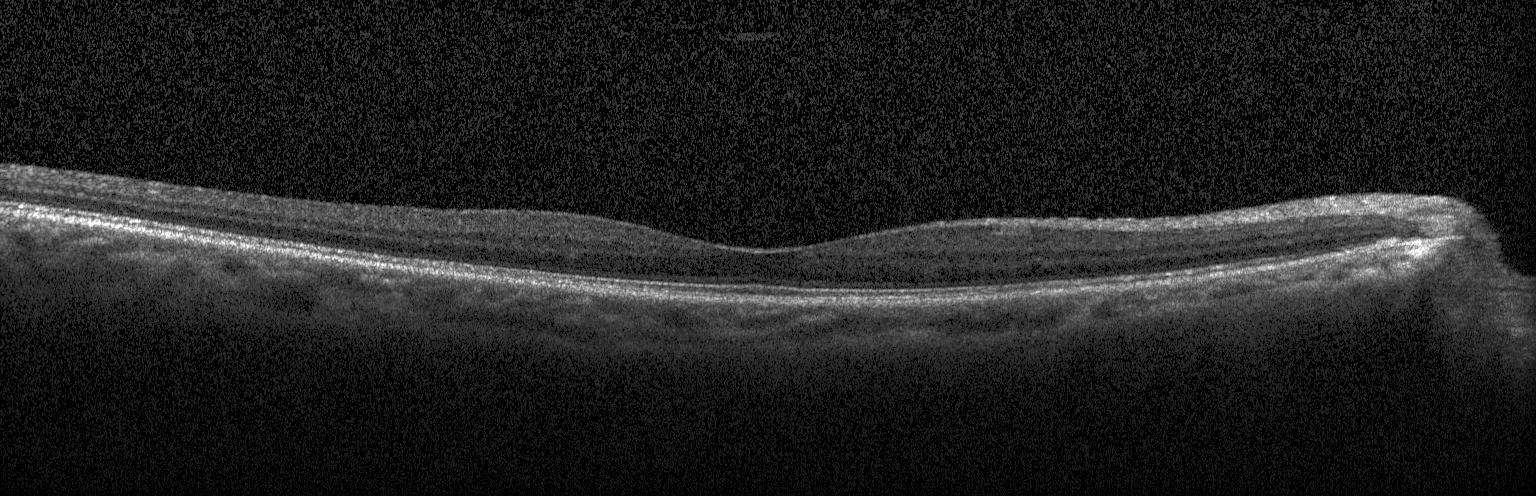
Retinal OCT B-scan. Fovea-centered. Heidelberg Spectralis OCT system
Finding: neither CNV, DME, nor drusen.